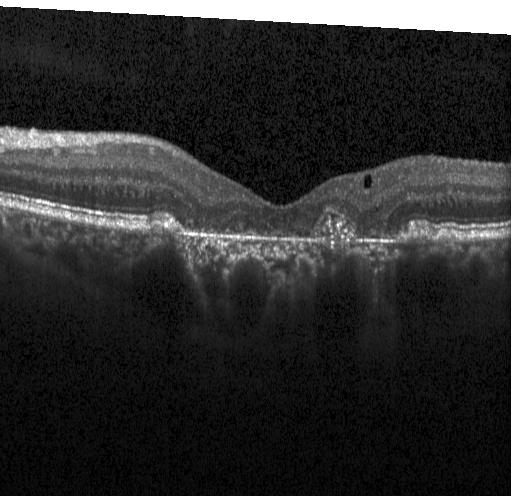 OCT B-scan · fovea-centered · Heidelberg Spectralis OCT system · SD-OCT — A choroidal neovascular membrane.